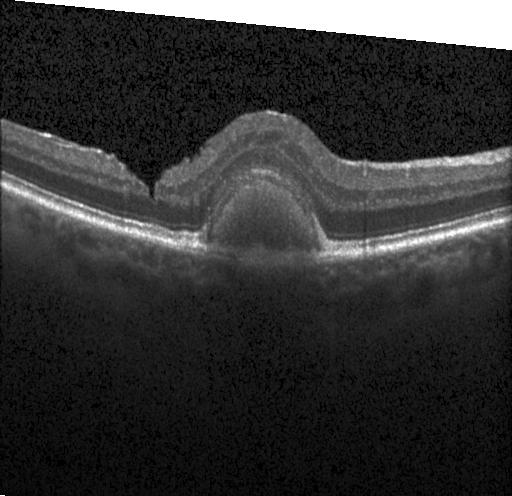
Centered on the fovea, retinal OCT cross-section. This B-scan demonstrates a choroidal neovascular membrane.